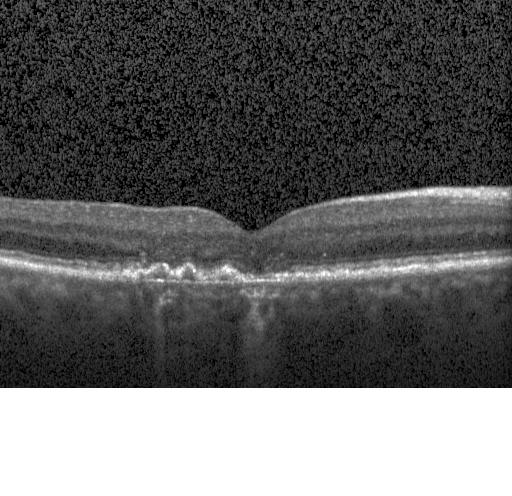
Retinal OCT cross-section — Diagnosis: choroidal neovascularization (CNV).